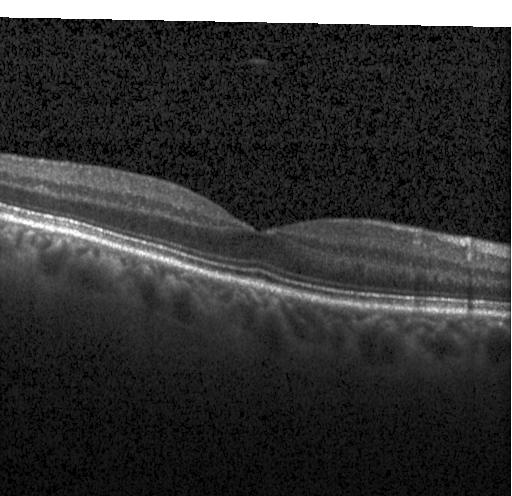
Instrument: Heidelberg Spectralis, retinal OCT B-scan, centered on the fovea, SD-OCT. OCT finding: no choroidal neovascularization, diabetic macular edema, or drusen.